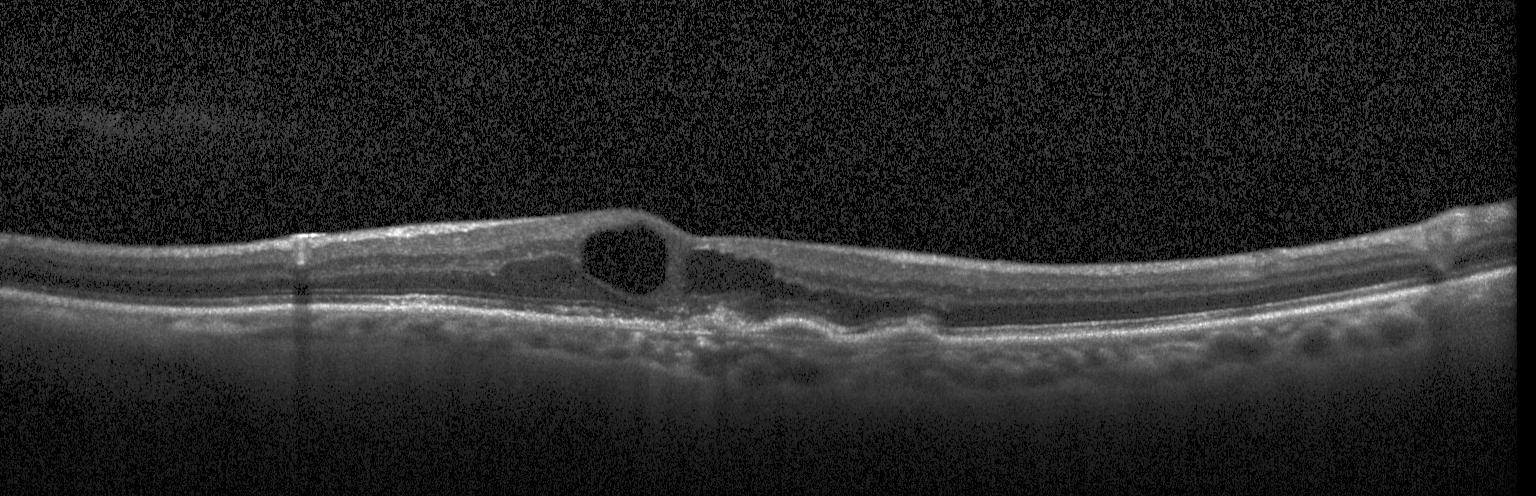

Assessment: CNV.